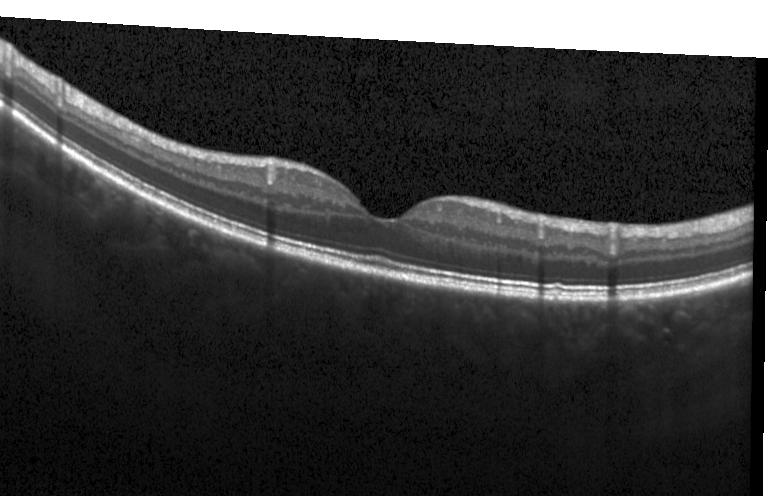 Macular scan; spectral-domain OCT; OCT line scan; Heidelberg Spectralis — Assessment: no choroidal neovascularization, no diabetic macular edema, and no drusen.